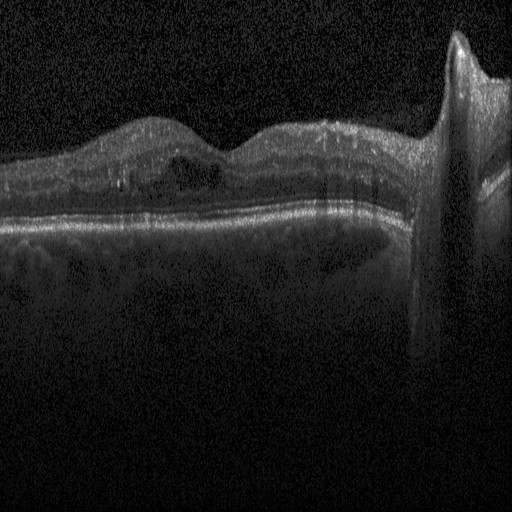 Finding: DME.